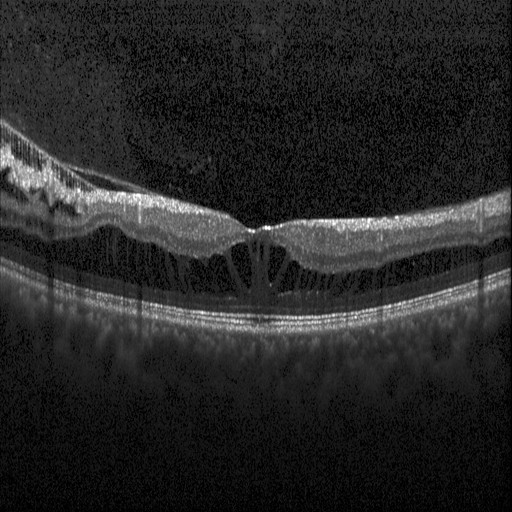 OCT line scan. Heidelberg Spectralis OCT system
Impression: diabetic macular edema.